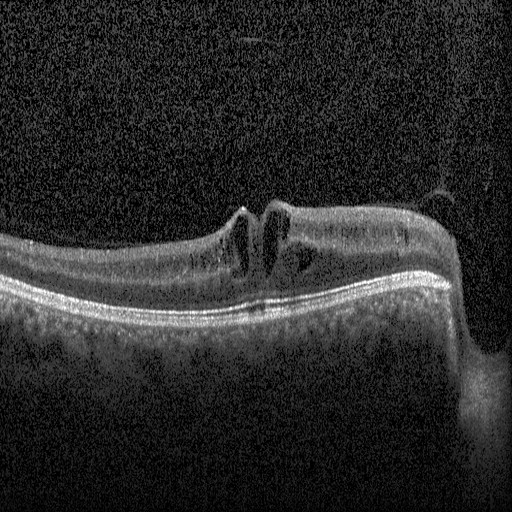
OCT line scan; spectral-domain OCT; instrument: Heidelberg Spectralis; macular scan. Dx: DME.